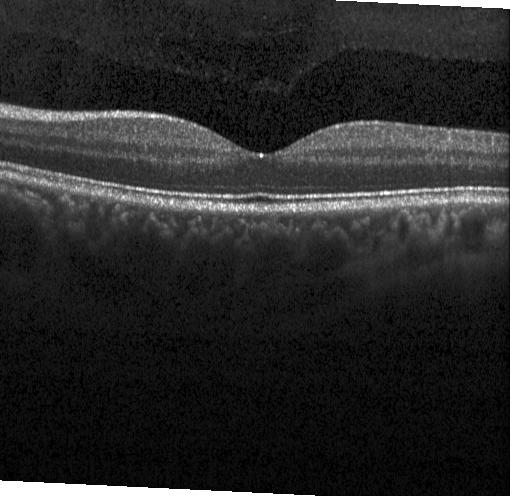

OCT finding: neither choroidal neovascularization, diabetic macular edema, nor drusen.